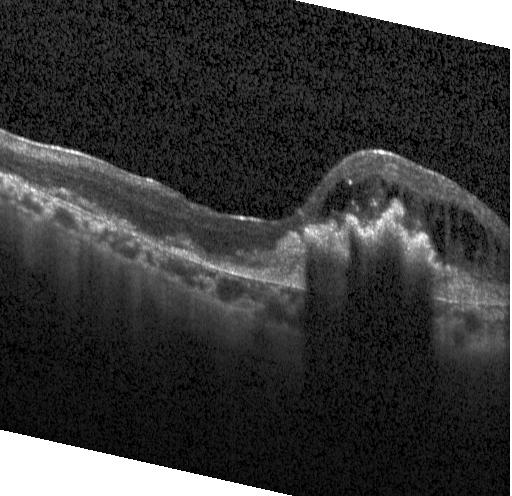

SD-OCT; retinal OCT cross-section. OCT finding: a choroidal neovascular membrane.